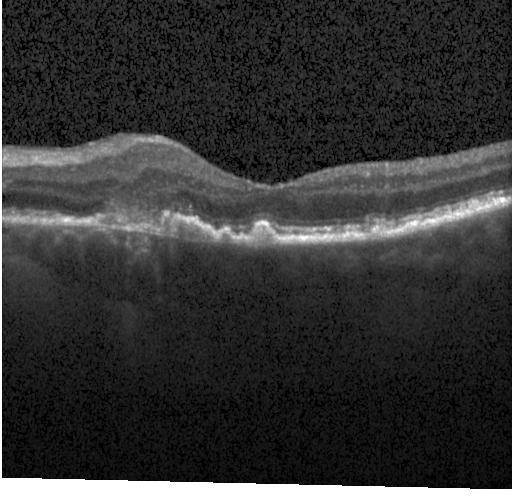
Heidelberg Spectralis; retinal OCT B-scan; SD-OCT; centered on the fovea. Finding: choroidal neovascularization (CNV).